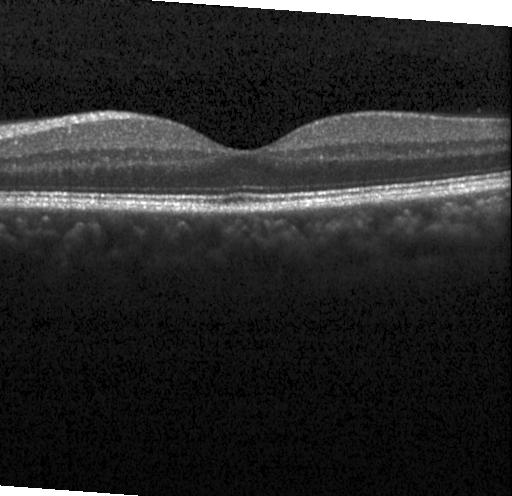
OCT line scan, Heidelberg Spectralis, horizontal scan through the fovea, spectral-domain optical coherence tomography
OCT finding: neither CNV, DME, nor drusen.